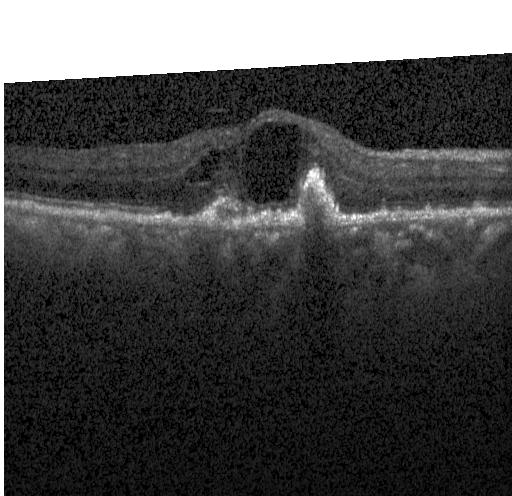

Impression: CNV.